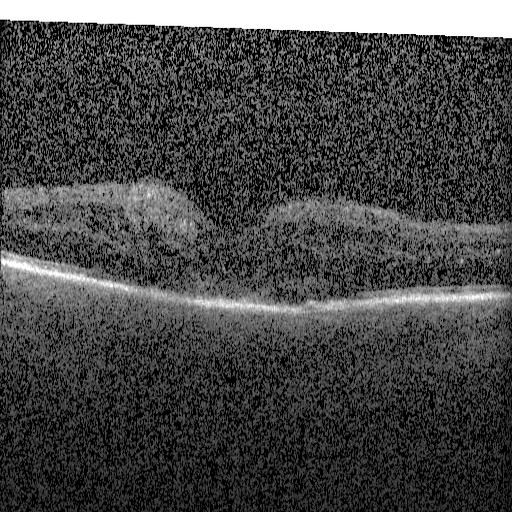 Retinal OCT cross-section. SD-OCT. Instrument: Heidelberg Spectralis.
Impression: diabetic macular edema.